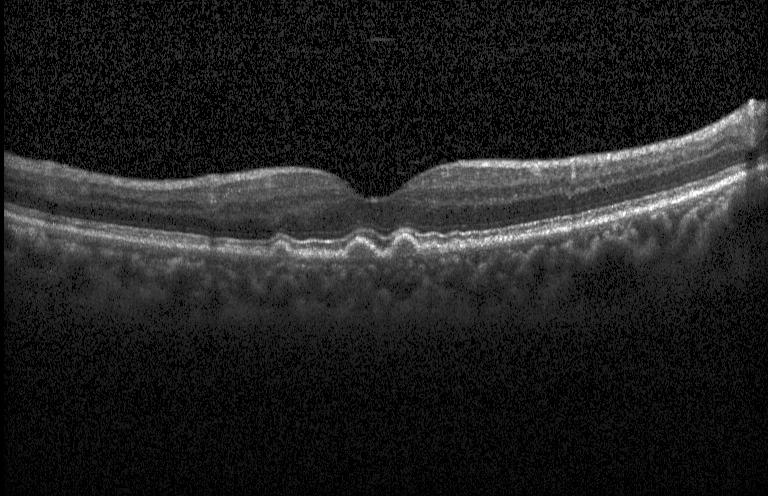

Centered on the fovea, Heidelberg Spectralis, retinal OCT cross-section, spectral-domain OCT — Impression: drusen.